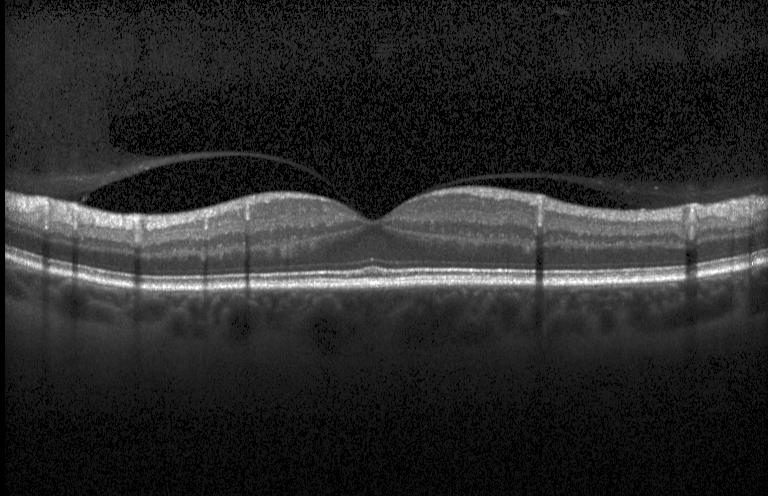
Spectral-domain OCT. Retinal OCT B-scan — Diagnosis: no evidence of CNV, DME, or drusen.